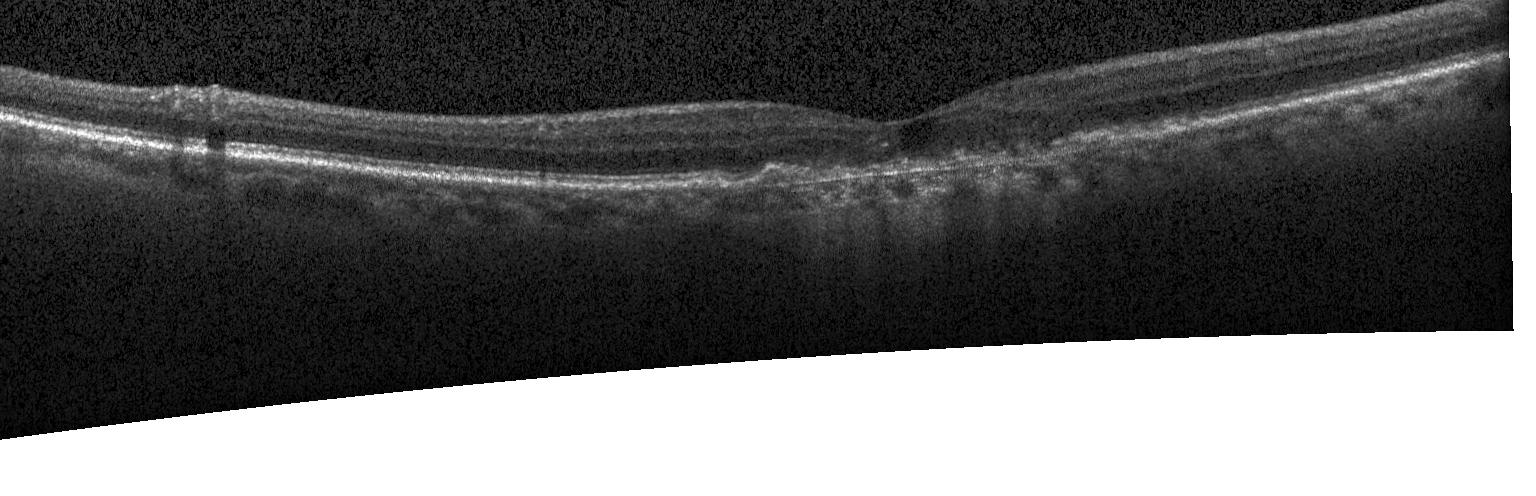
Optical coherence tomography scan. Instrument: Heidelberg Spectralis. Spectral-domain optical coherence tomography.
Diagnosis: CNV.